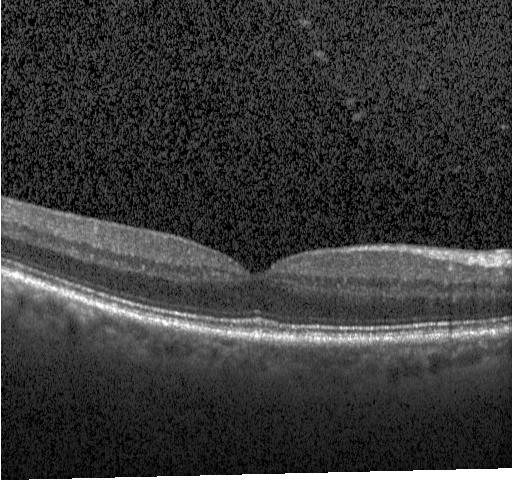

Macular OCT: no choroidal neovascularization, no diabetic macular edema, and no drusen.